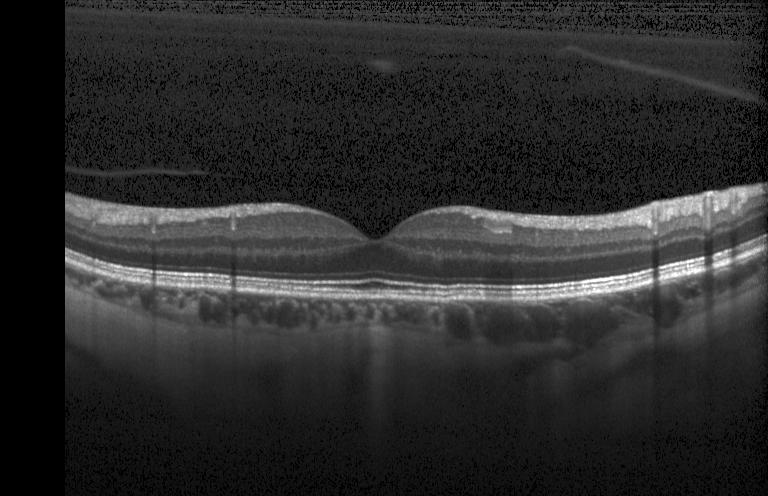 Through the macula, optical coherence tomography scan
Neither choroidal neovascularization, diabetic macular edema, nor drusen.